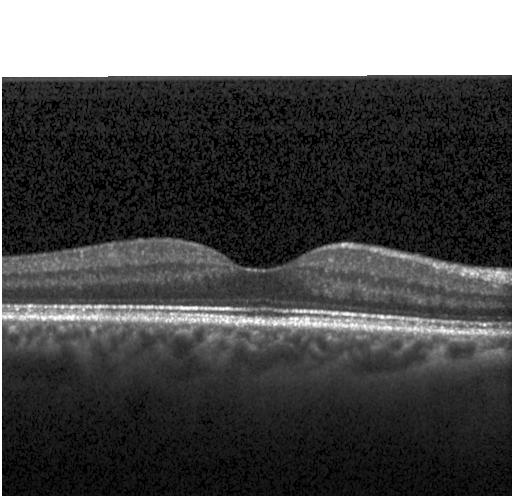
Heidelberg Spectralis; OCT line scan.
OCT finding: no choroidal neovascularization, no diabetic macular edema, and no drusen.